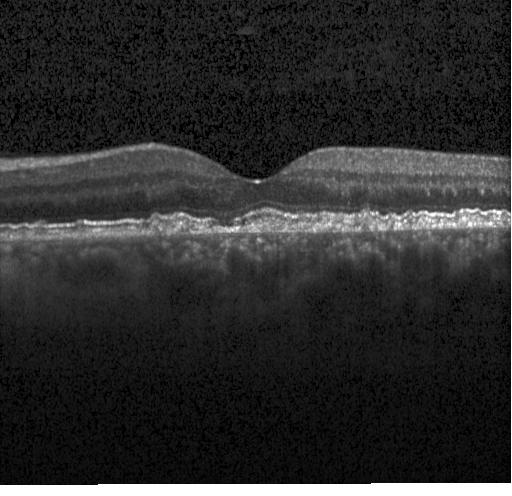

Dx: drusen.